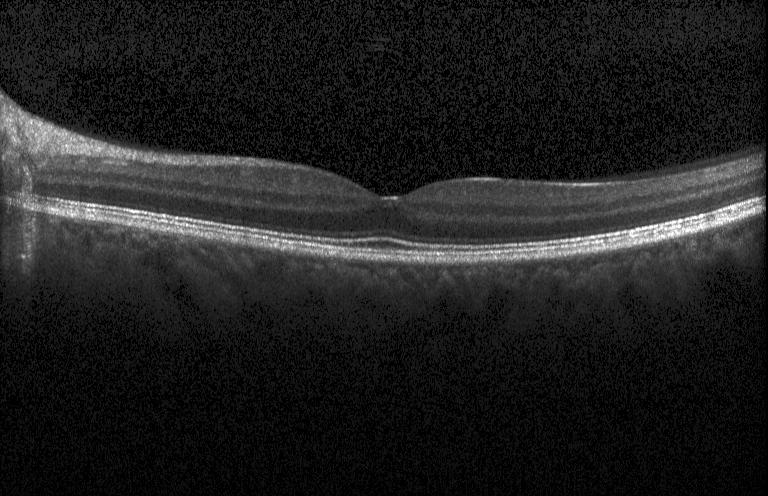 Impression: no choroidal neovascularization, no diabetic macular edema, and no drusen.